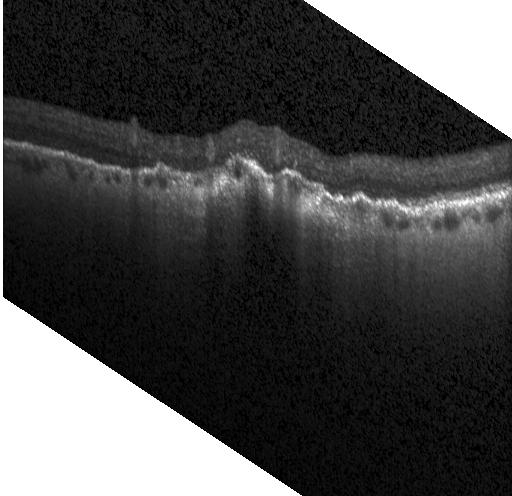

Centered on the fovea. Retinal OCT cross-section. SD-OCT
Impression: choroidal neovascularization.